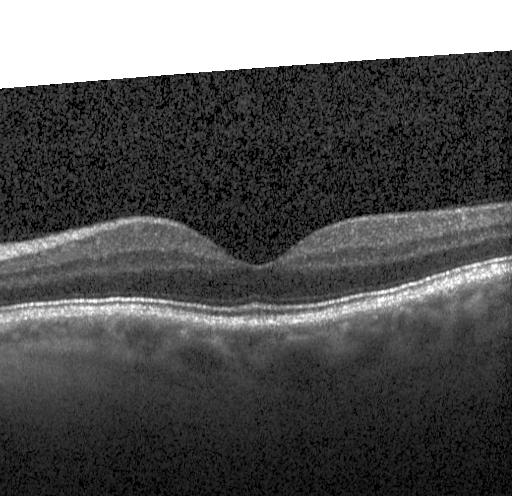
Finding: neither choroidal neovascularization, diabetic macular edema, nor drusen.